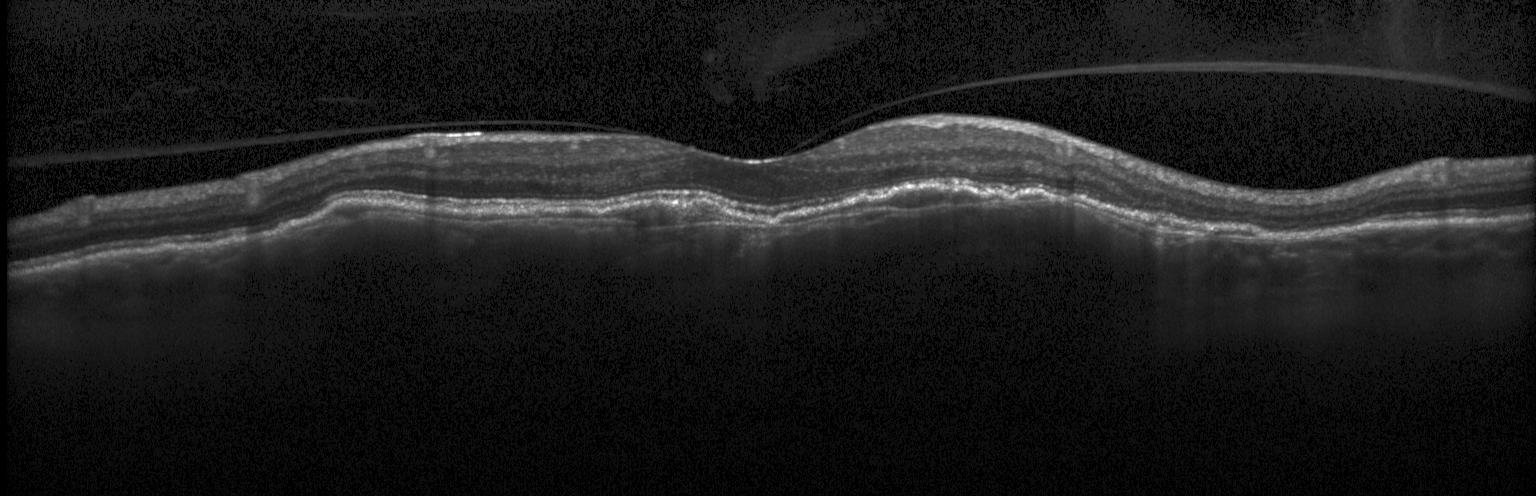
OCT line scan; Heidelberg Spectralis; horizontal scan through the fovea; SD-OCT
Finding: a choroidal neovascular membrane.